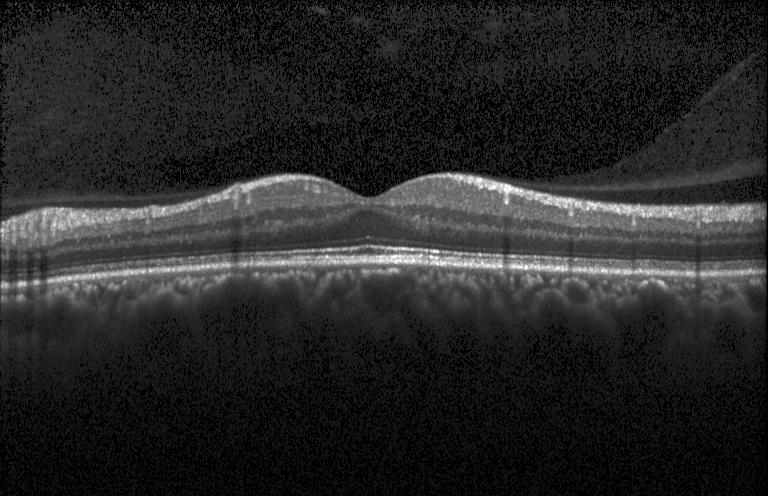
Spectral-domain OCT · OCT B-scan · horizontal scan through the fovea · instrument: Heidelberg Spectralis.
Assessment: no evidence of choroidal neovascularization, diabetic macular edema, or drusen.